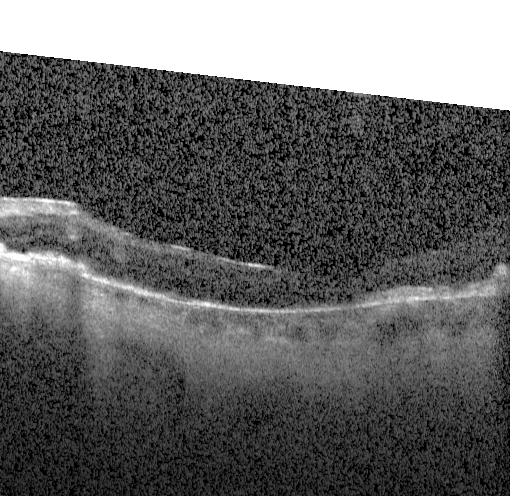

Macular OCT: CNV.